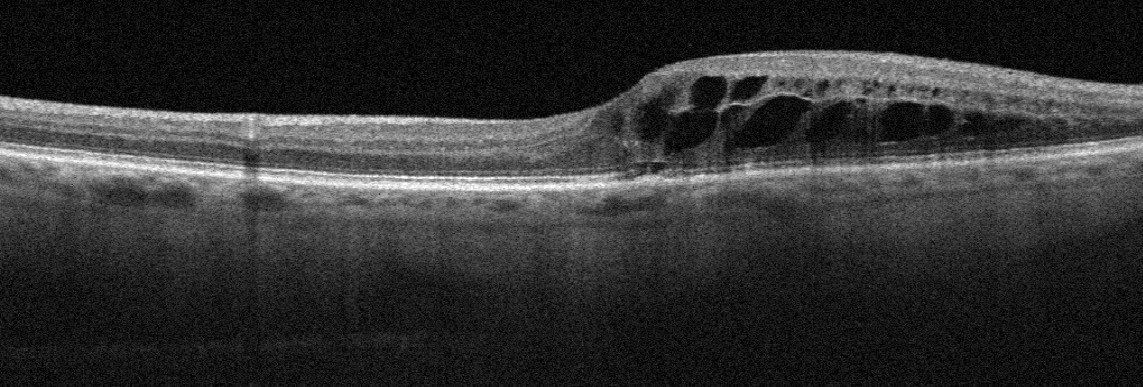

Acquired on an Optovue Avanti RTVue XR; optical coherence tomography scan; macular scan. OCT finding: RVO.